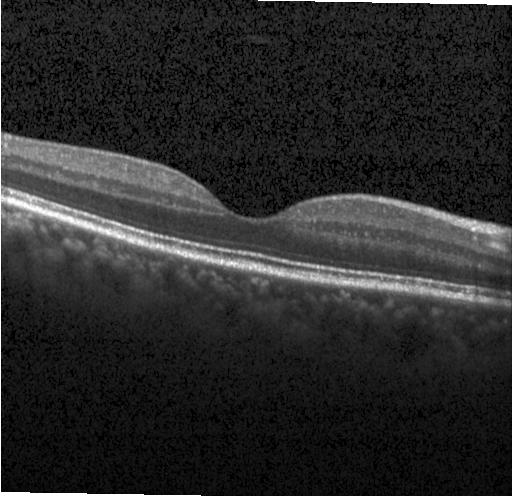 Assessment: no CNV, DME, or drusen.